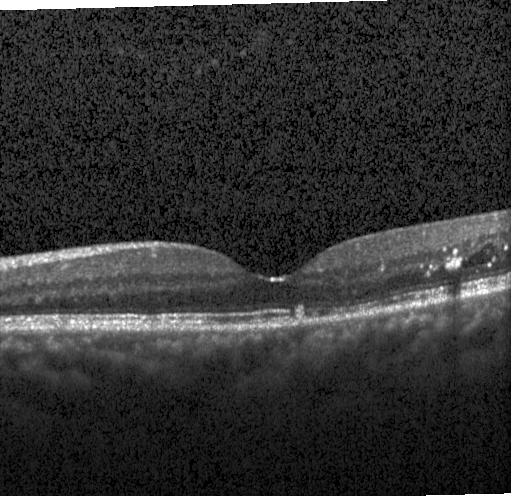 Retinal OCT cross-section showing diabetic macular edema.